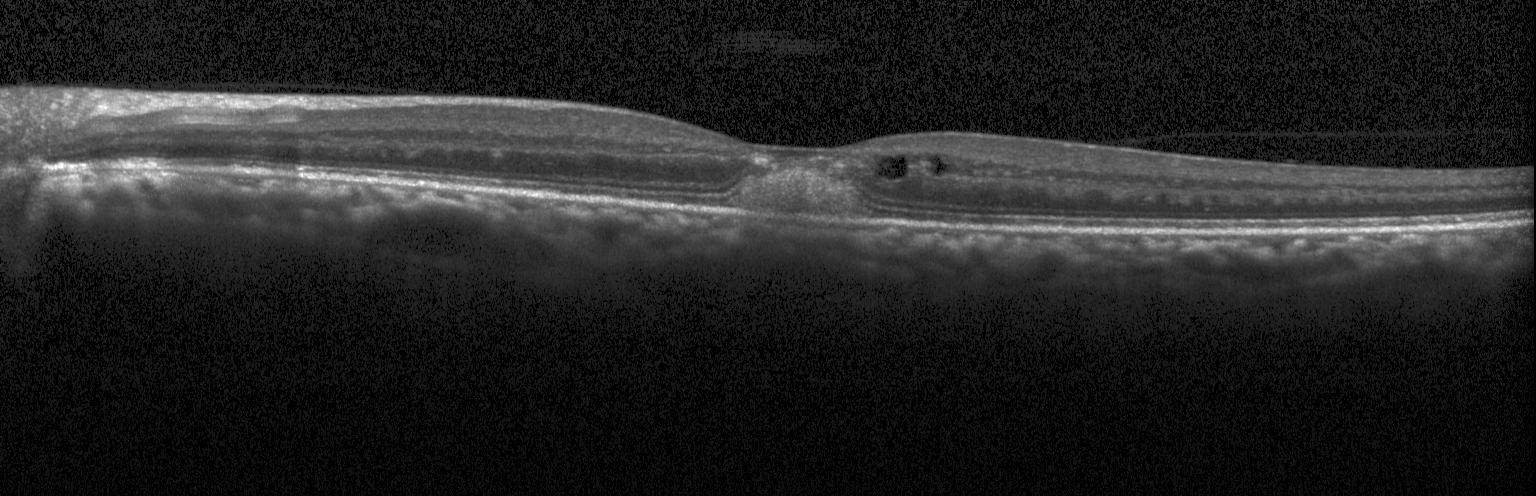

This B-scan demonstrates choroidal neovascularization.